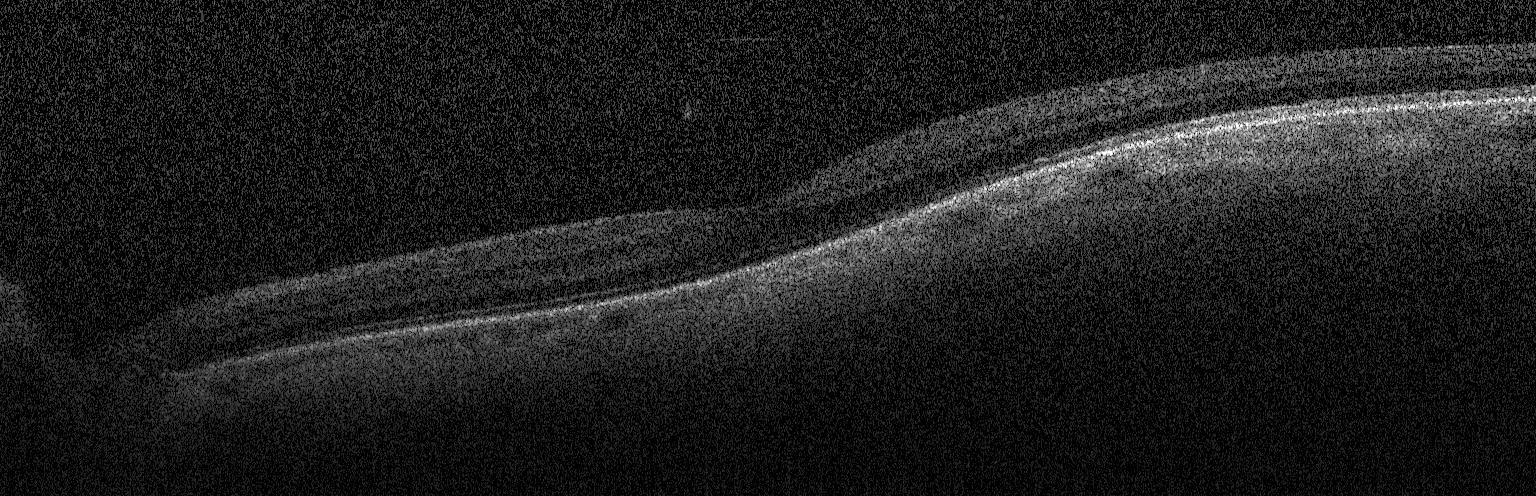 Retinal OCT cross-section; horizontal scan through the fovea; spectral-domain OCT
Impression: neither choroidal neovascularization, diabetic macular edema, nor drusen.